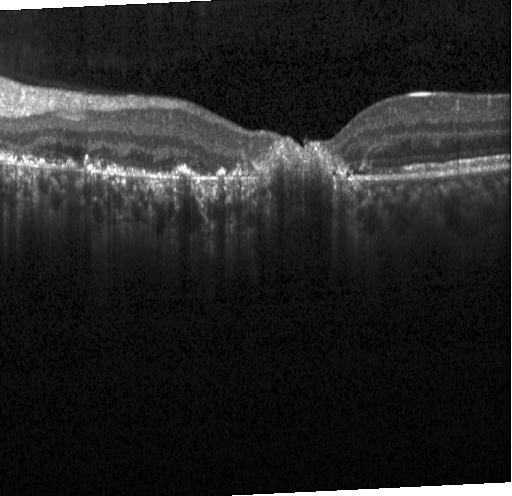
Dx: choroidal neovascularization (CNV).